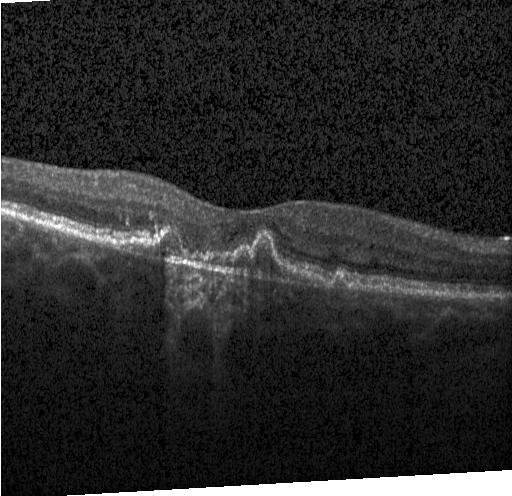
OCT line scan; centered on the fovea. Diagnosis: a choroidal neovascular membrane.